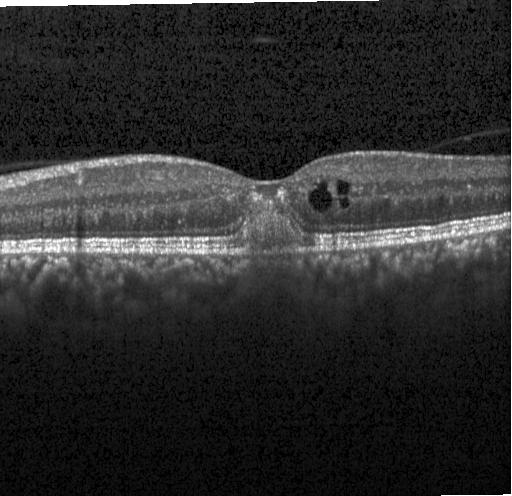

Retinal OCT B-scan. Choroidal neovascularization (CNV).